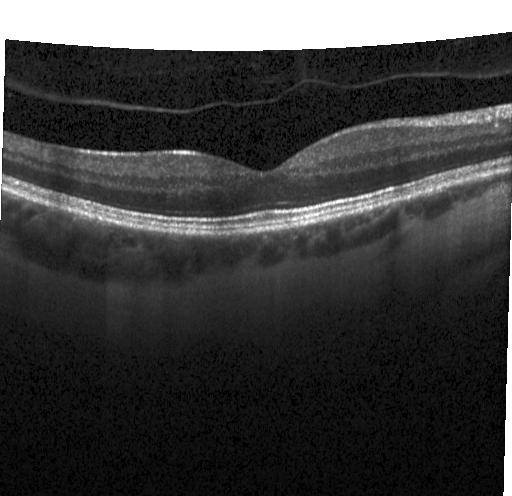
Spectral-domain OCT; optical coherence tomography scan; instrument: Heidelberg Spectralis.
The scan shows no evidence of choroidal neovascularization, diabetic macular edema, or drusen.